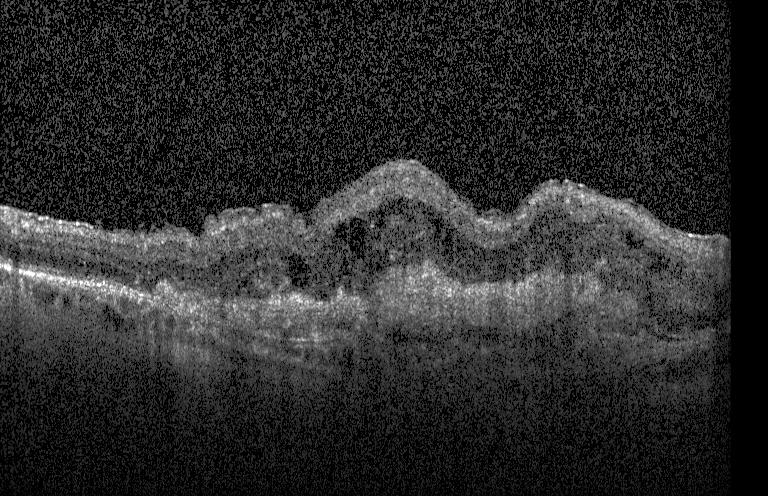 Impression: choroidal neovascularization (CNV).